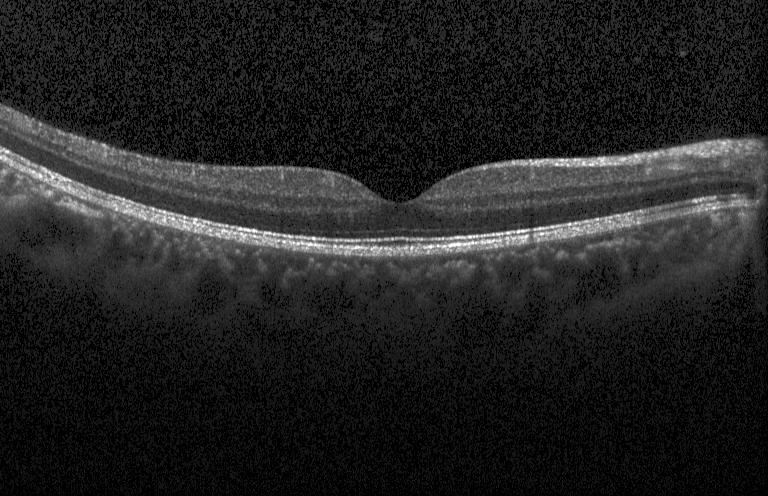

Retinal OCT B-scan — Diagnosis: no choroidal neovascularization, diabetic macular edema, or drusen.